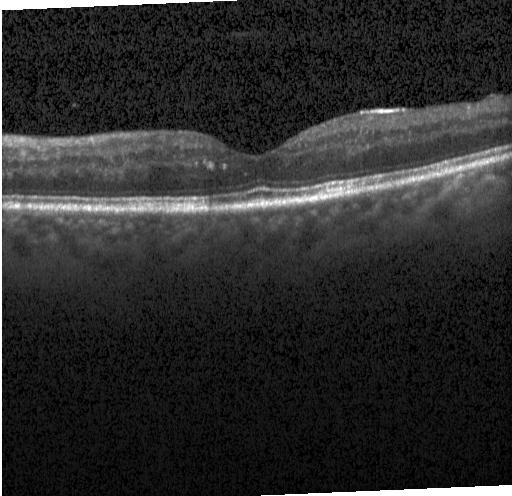 The scan shows no evidence of choroidal neovascularization, diabetic macular edema, or drusen.